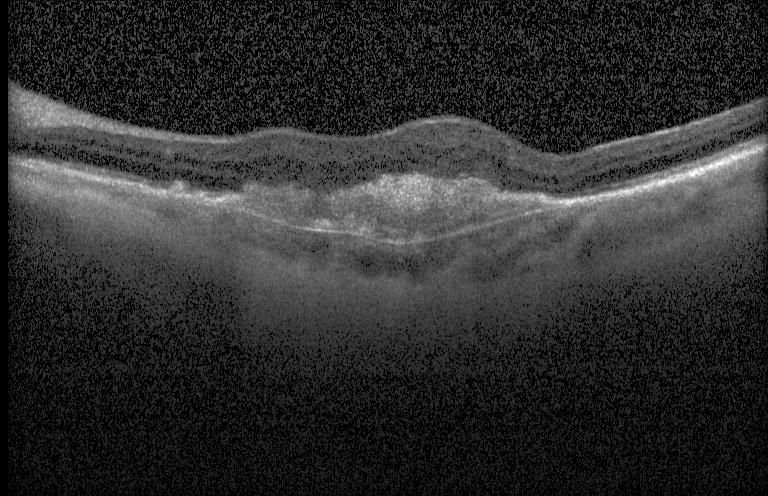

Macular OCT: choroidal neovascularization.